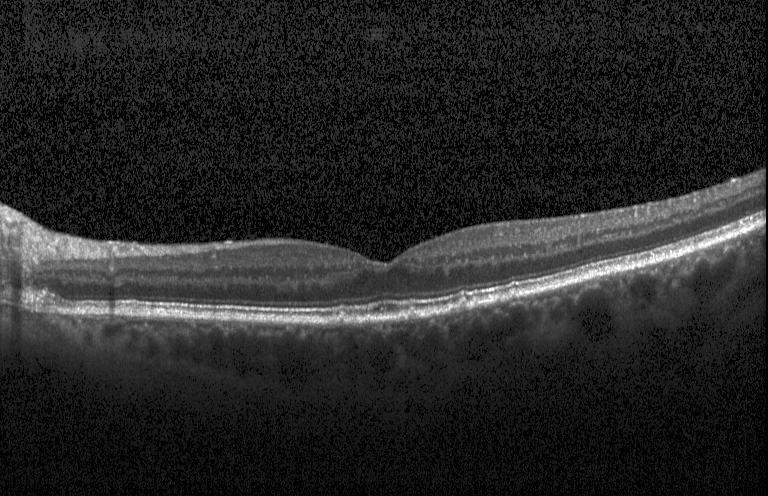 OCT line scan · acquired on a Heidelberg Spectralis · spectral-domain optical coherence tomography
Impression: drusen.